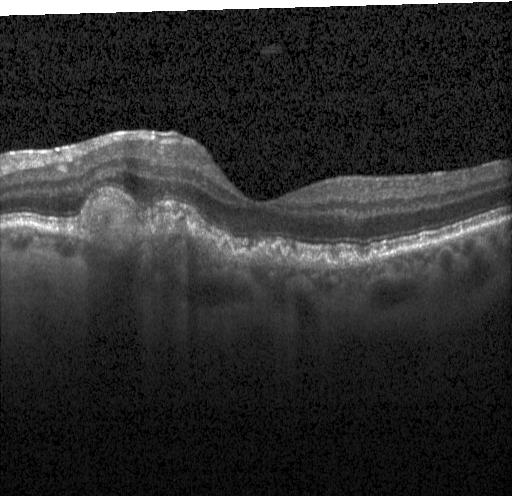
Retinal OCT B-scan · acquired on a Heidelberg Spectralis · SD-OCT — Impression: a choroidal neovascular membrane.